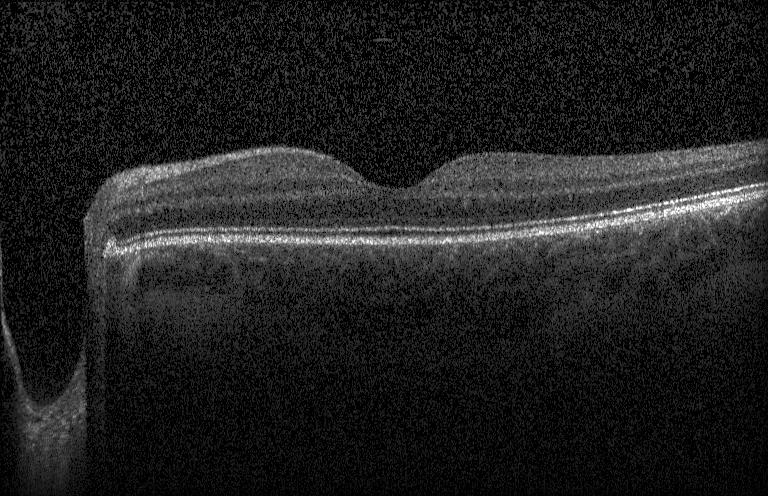

OCT finding: no CNV, DME, or drusen.